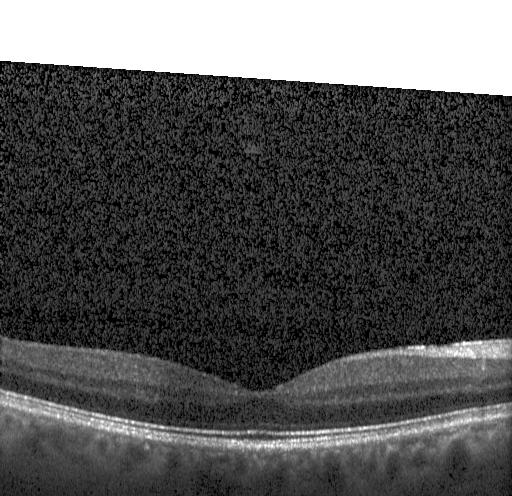

Spectral-domain OCT. Fovea-centered. Retinal OCT B-scan. Heidelberg Spectralis OCT system. This B-scan demonstrates no choroidal neovascularization, diabetic macular edema, or drusen.